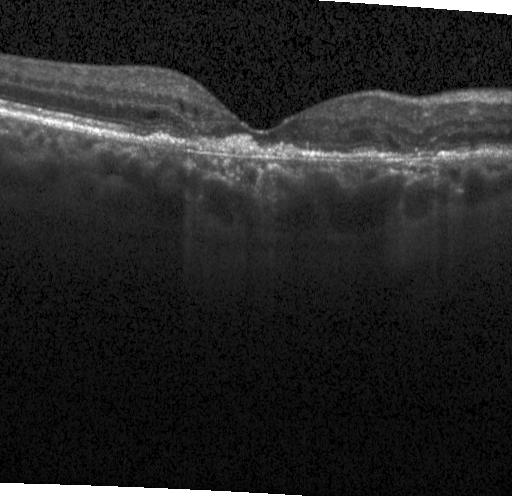 The scan shows CNV.